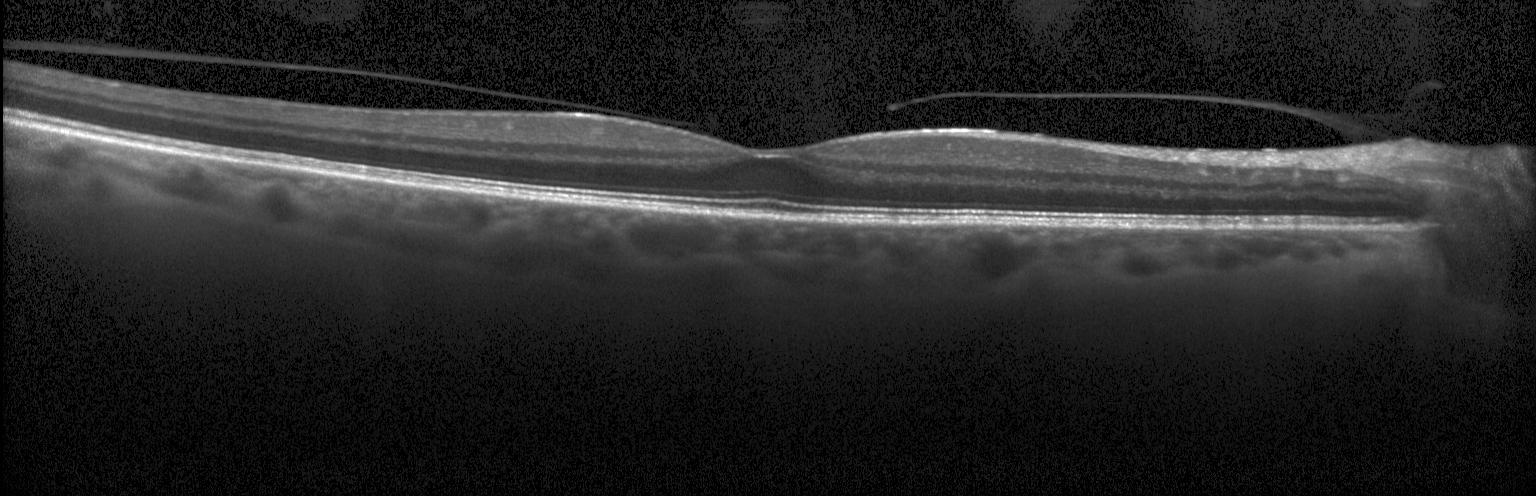 Horizontal scan through the fovea, optical coherence tomography B-scan. Dx: neither choroidal neovascularization, diabetic macular edema, nor drusen.